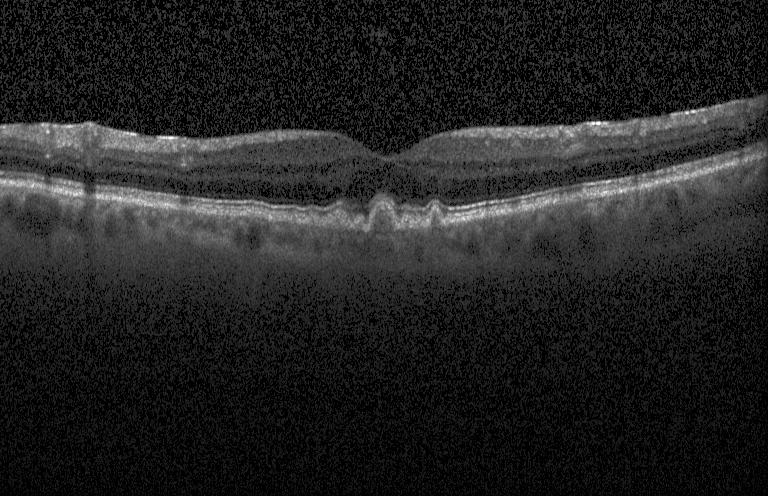
Centered on the fovea · instrument: Heidelberg Spectralis · optical coherence tomography scan. Dx: drusen.